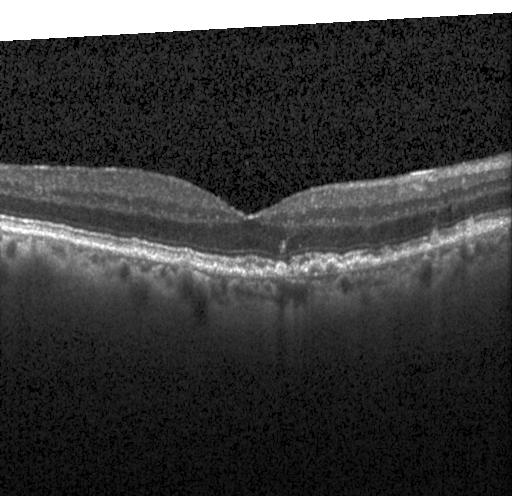 Macular OCT demonstrating multiple drusen.